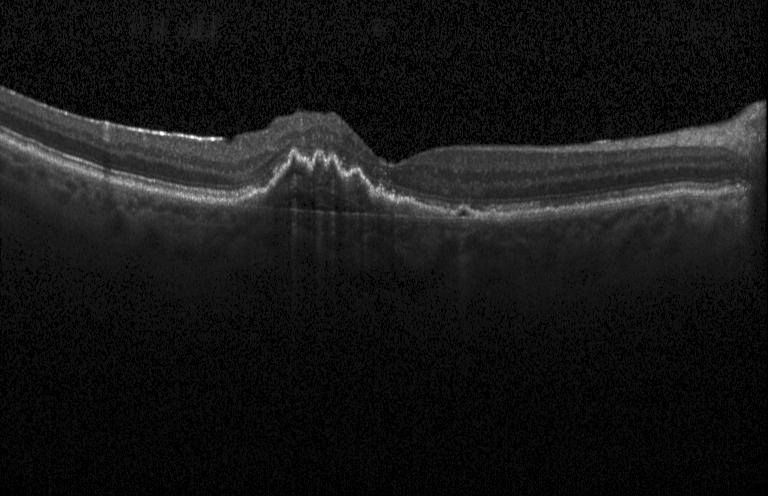

Retinal OCT B-scan
Diagnosis: a choroidal neovascular membrane.